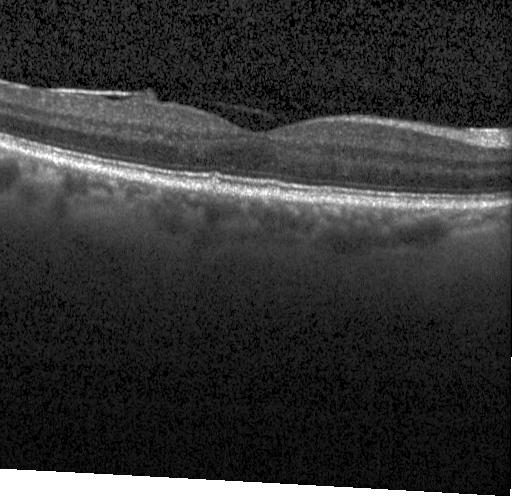 Retinal OCT B-scan
Finding: drusen.